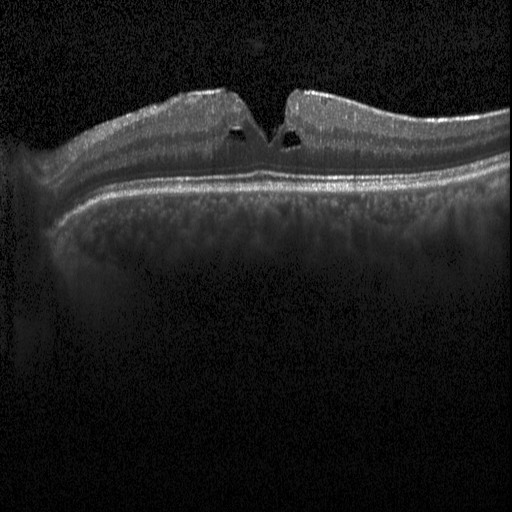 Spectral-domain OCT B-scan: diabetic macular edema.